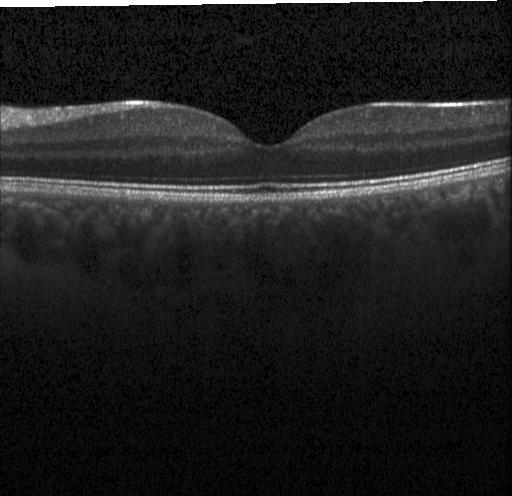
Finding: no evidence of choroidal neovascularization, diabetic macular edema, or drusen.